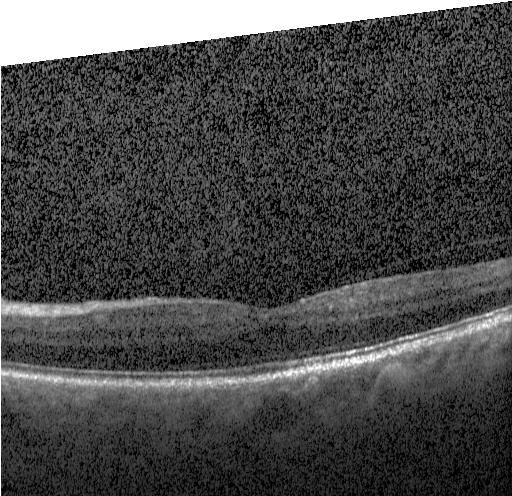
Assessment: no choroidal neovascularization, diabetic macular edema, or drusen.